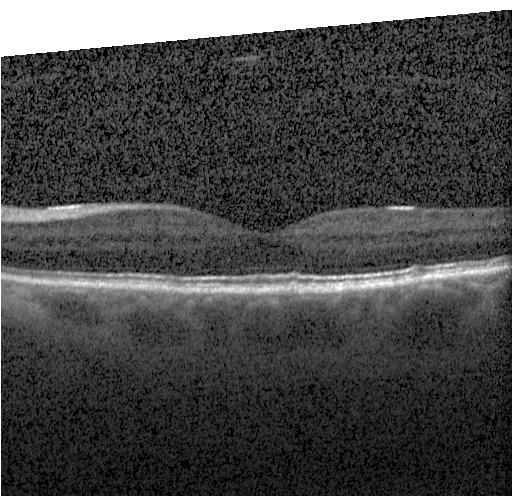

Retinal OCT B-scan; through the macula; spectral-domain optical coherence tomography; acquired on a Heidelberg Spectralis. The scan shows multiple drusen.